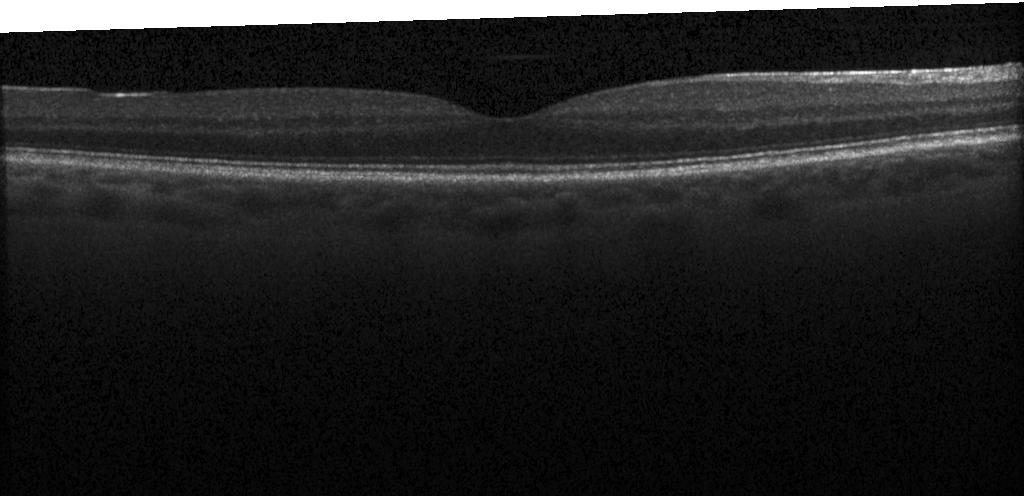

Optical coherence tomography B-scan, through the macula
Finding: no evidence of choroidal neovascularization, diabetic macular edema, or drusen.